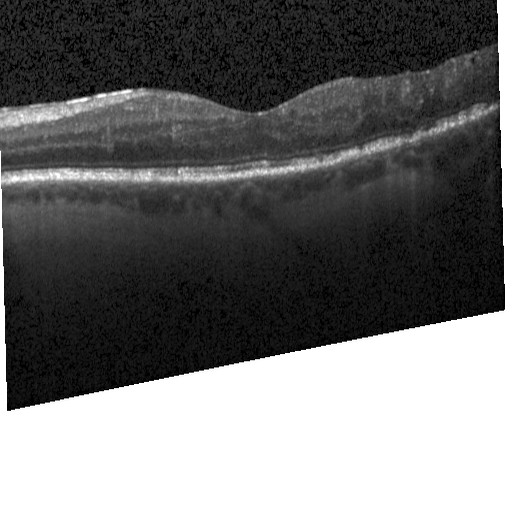
Impression: diabetic macular edema.